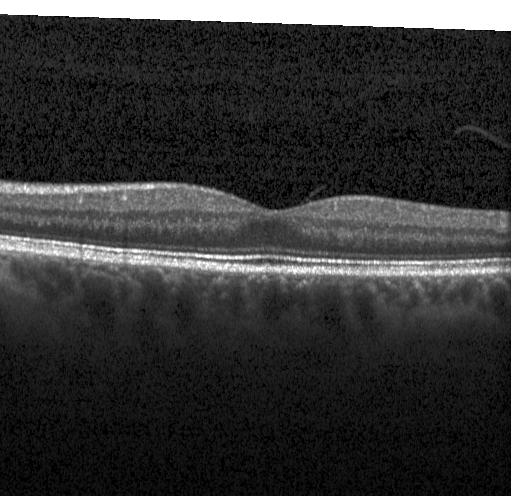 Optical coherence tomography B-scan.
Dx: neither choroidal neovascularization, diabetic macular edema, nor drusen.